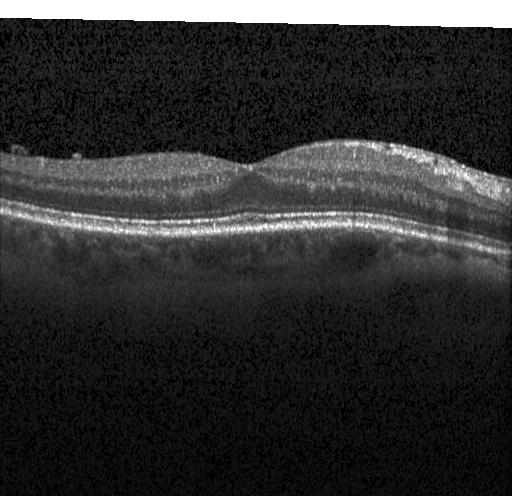

Retinal OCT B-scan
Impression: no CNV, DME, or drusen.